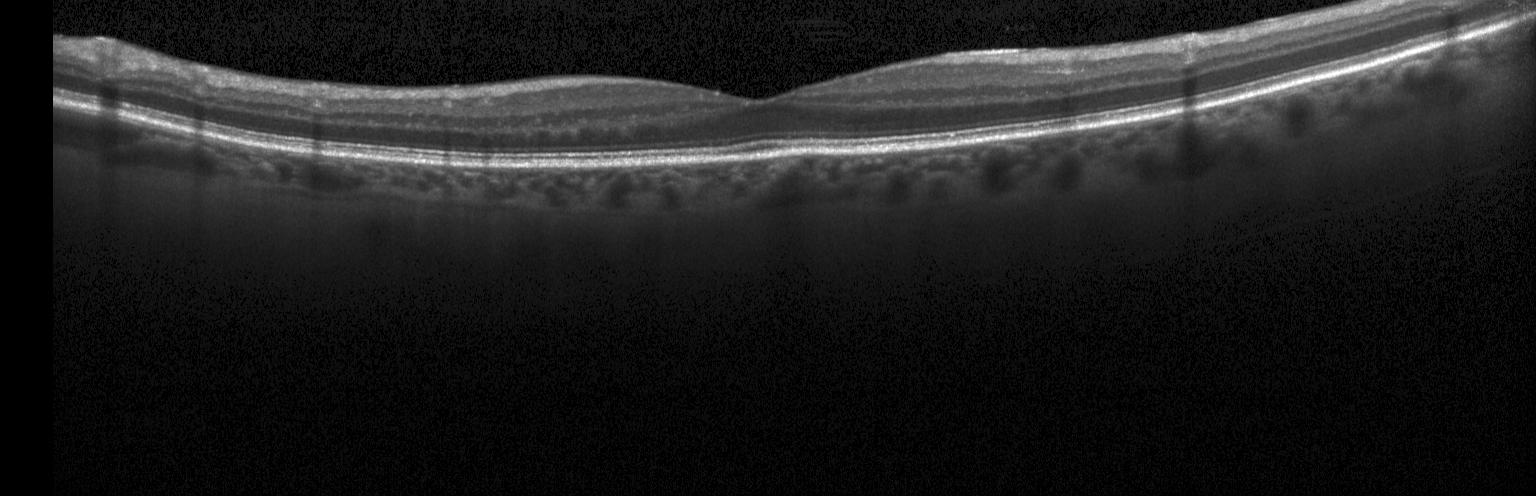
Optical coherence tomography scan. Heidelberg Spectralis.
Impression: no choroidal neovascularization, no diabetic macular edema, and no drusen.